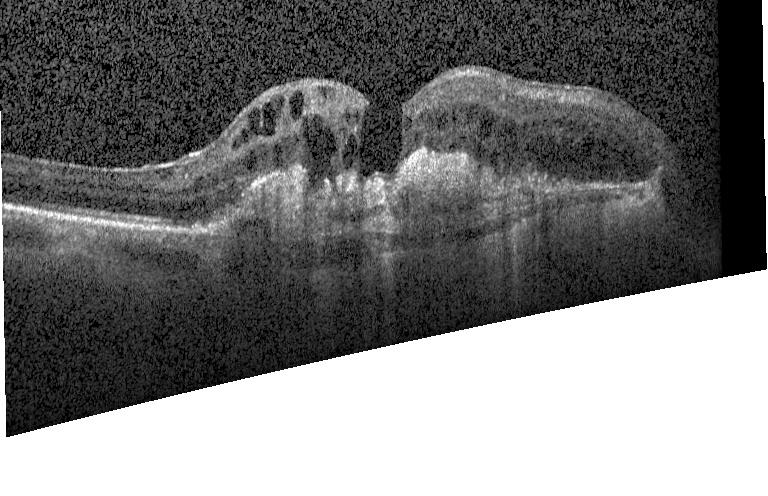

Dx: CNV.